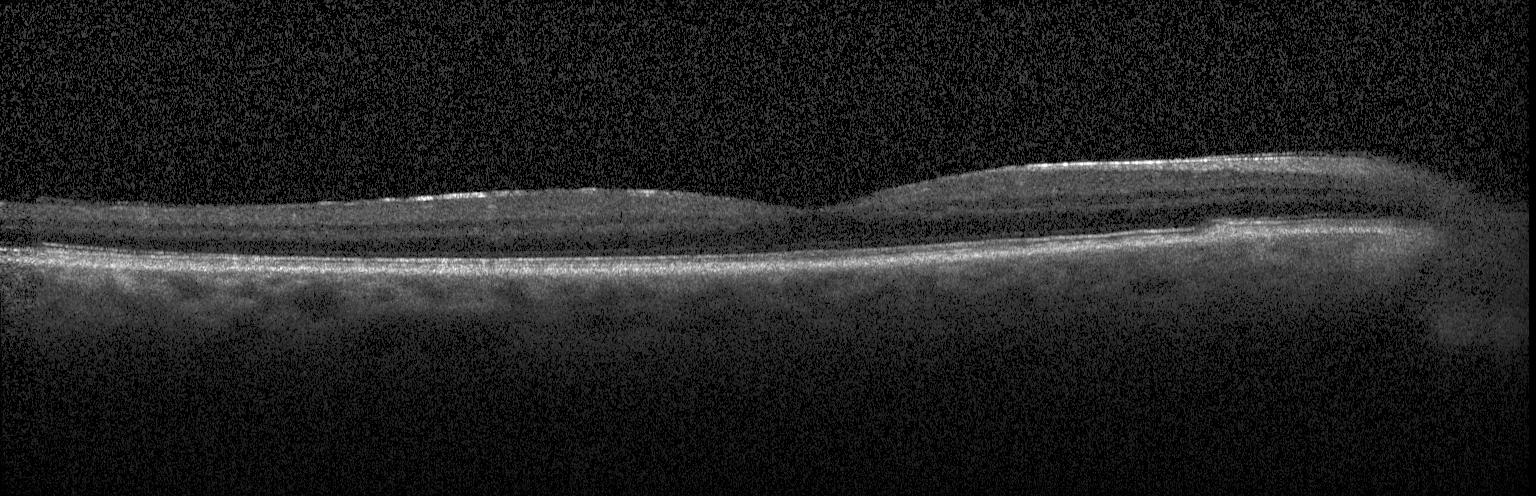 Instrument: Heidelberg Spectralis, retinal OCT cross-section. Assessment: neither choroidal neovascularization, diabetic macular edema, nor drusen.